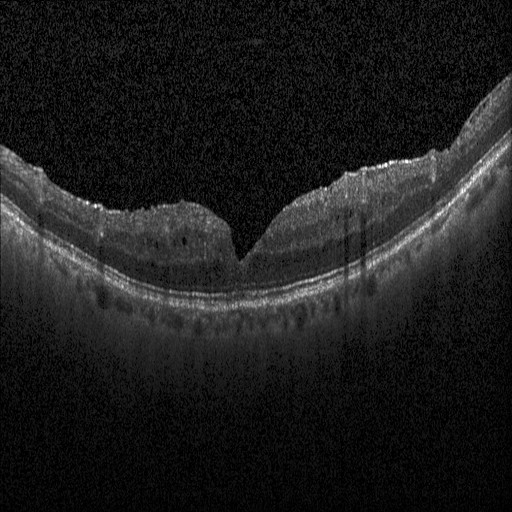
Fovea-centered; retinal OCT B-scan.
Dx: DME.